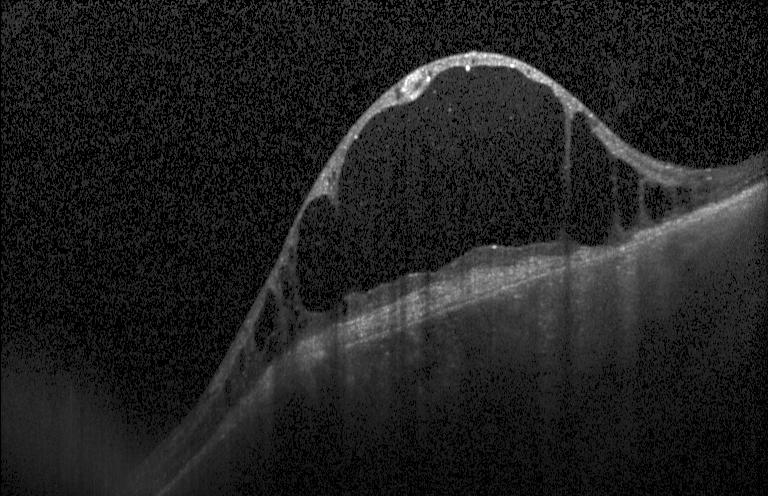 Dx: a choroidal neovascular membrane.